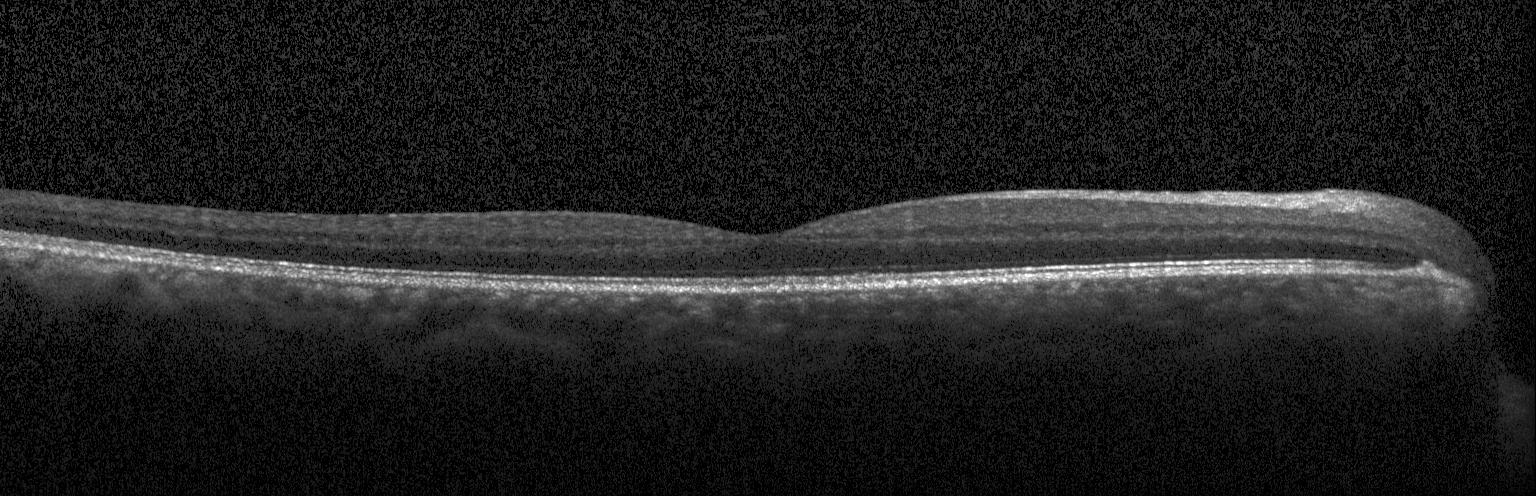

Retinal OCT B-scan — Finding: no CNV, no DME, and no drusen.